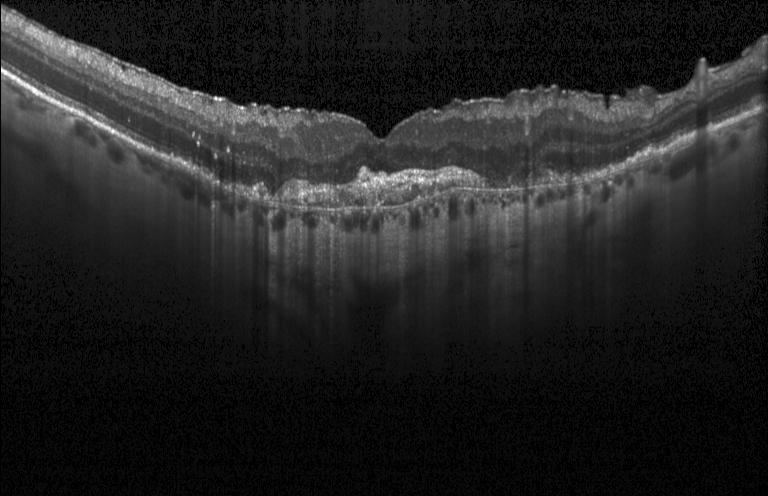 Retinal OCT cross-section.
Finding: a choroidal neovascular membrane.